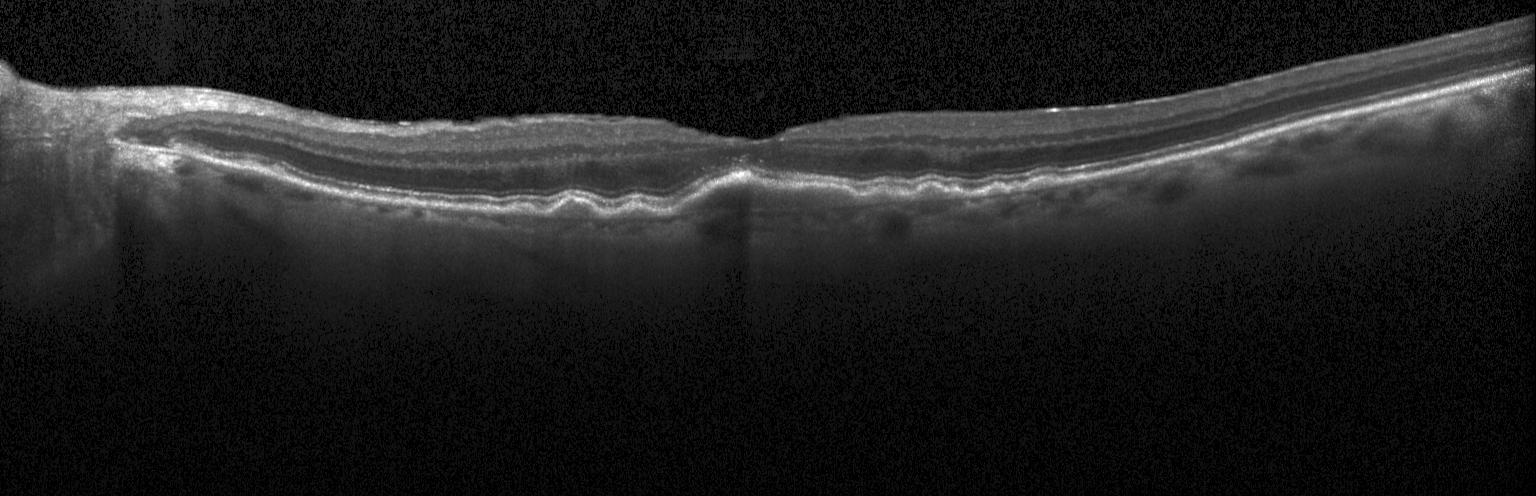 Impression: a choroidal neovascular membrane.